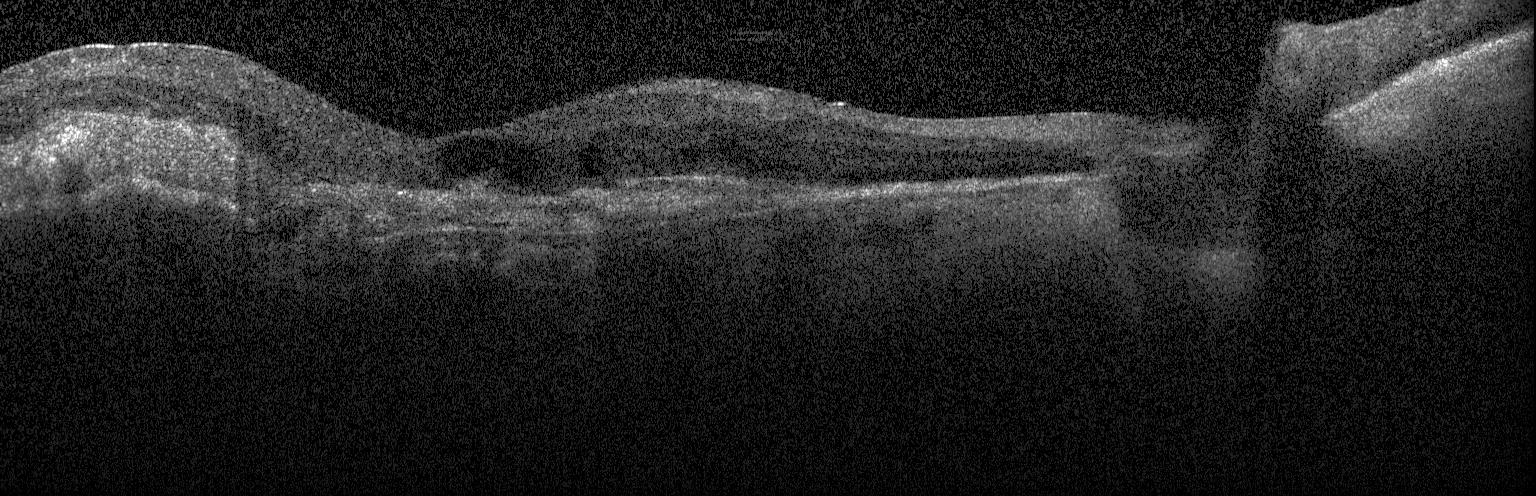
Heidelberg Spectralis, retinal OCT B-scan, macular scan, spectral-domain optical coherence tomography.
Diagnosis: choroidal neovascularization.